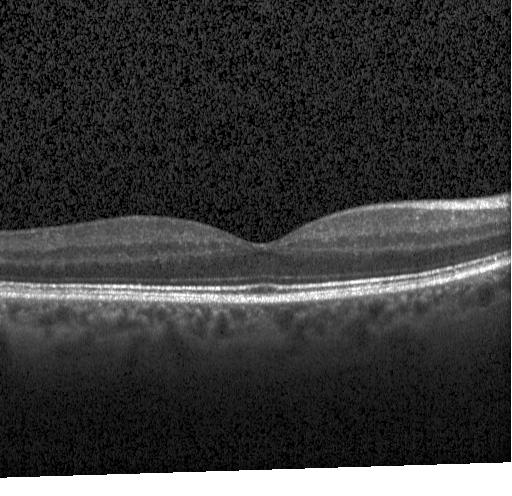
OCT scan showing no evidence of CNV, DME, or drusen.